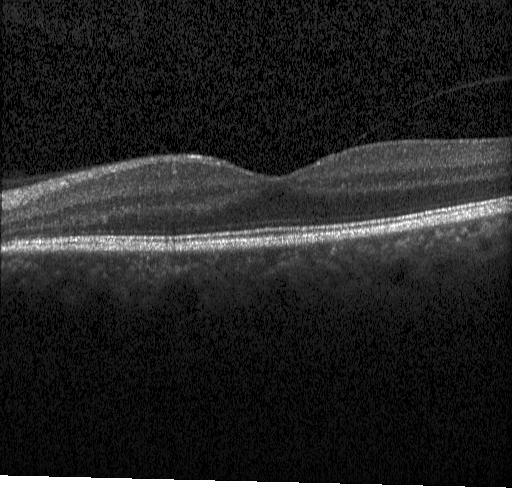

Through the macula; optical coherence tomography B-scan — Finding: no evidence of CNV, DME, or drusen.